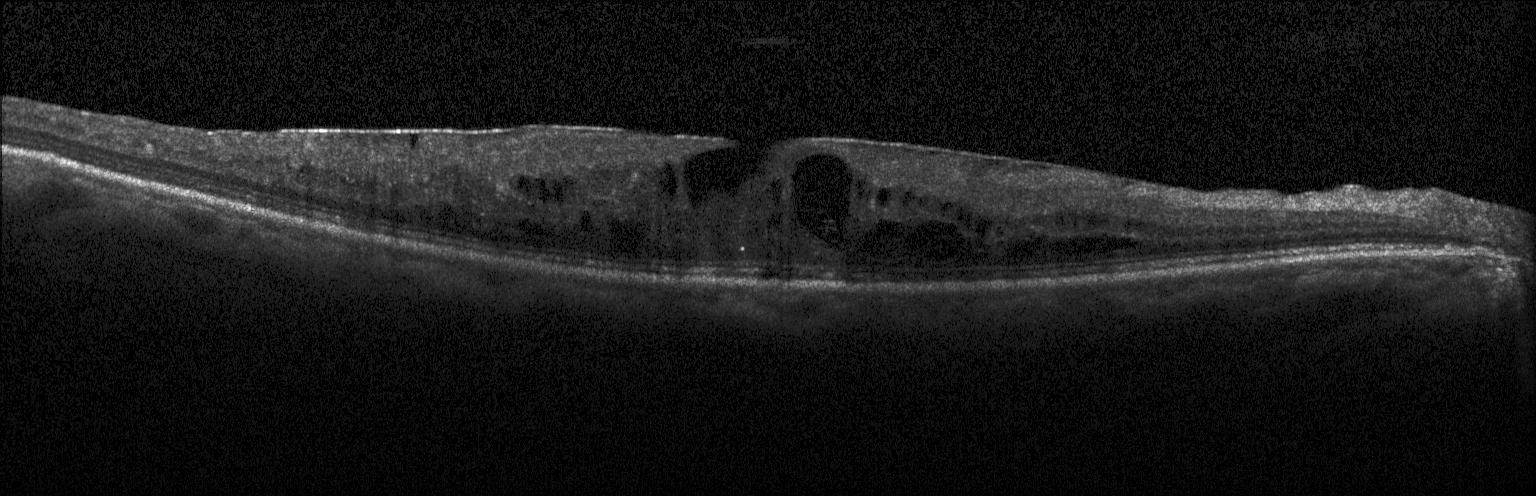 Retinal OCT B-scan, Heidelberg Spectralis
Diagnosis: diabetic macular edema.